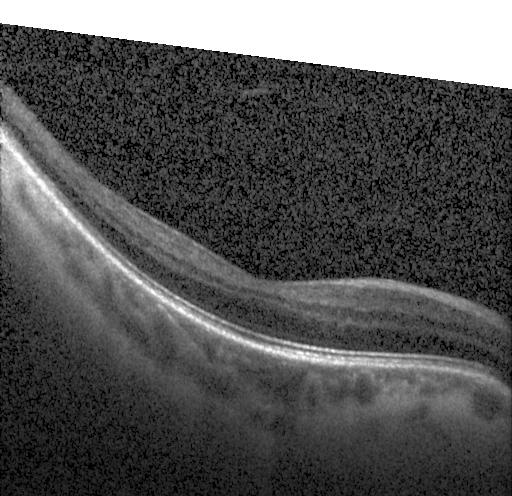

OCT line scan
Impression: no CNV, DME, or drusen.